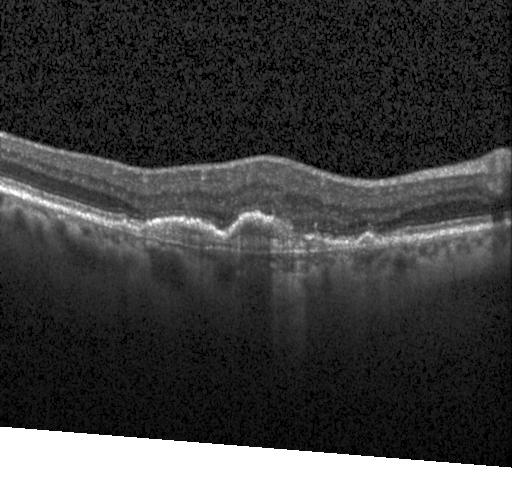
Optical coherence tomography scan; centered on the fovea; Heidelberg Spectralis — This B-scan demonstrates a choroidal neovascular membrane.